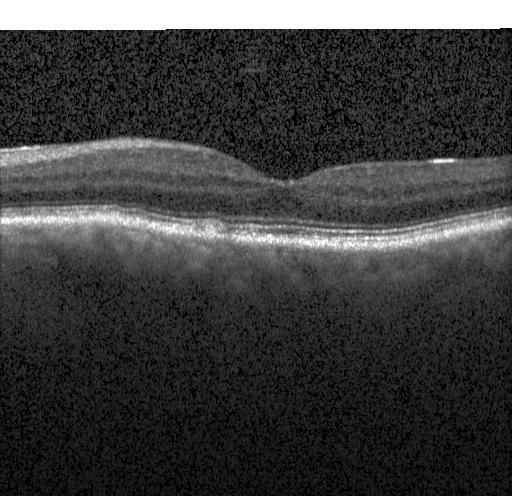 Centered on the fovea; spectral-domain OCT; OCT B-scan; Heidelberg Spectralis
Impression: sub-RPE drusenoid deposits.